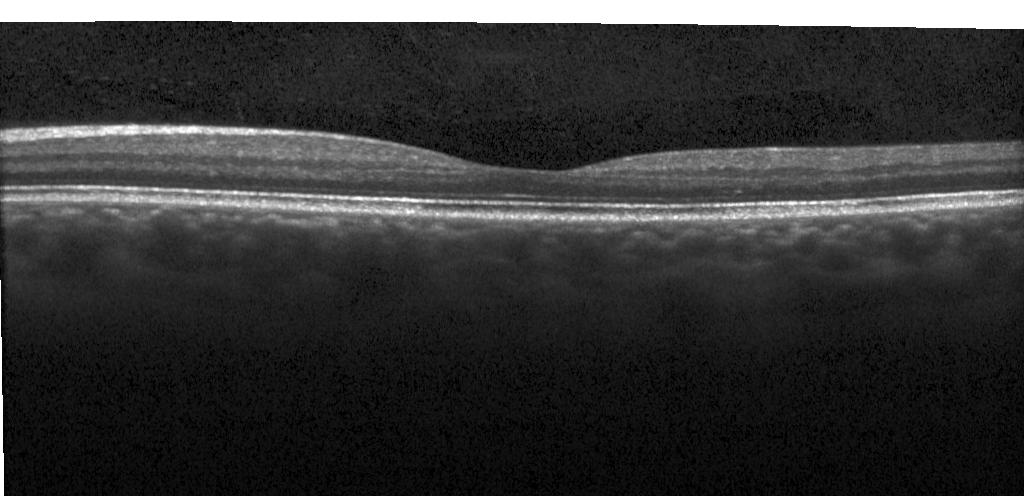
OCT scan showing no CNV, DME, or drusen.